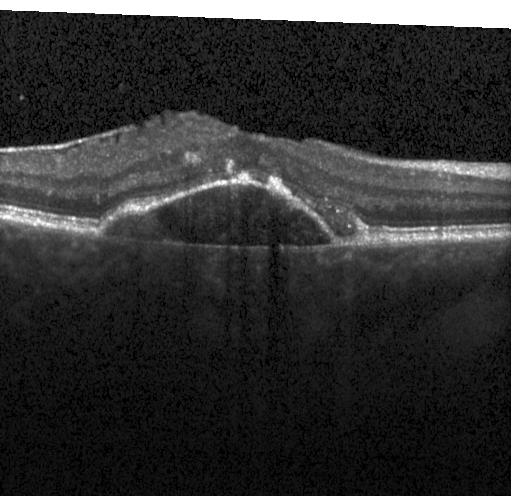 Spectral-domain OCT B-scan: a choroidal neovascular membrane.